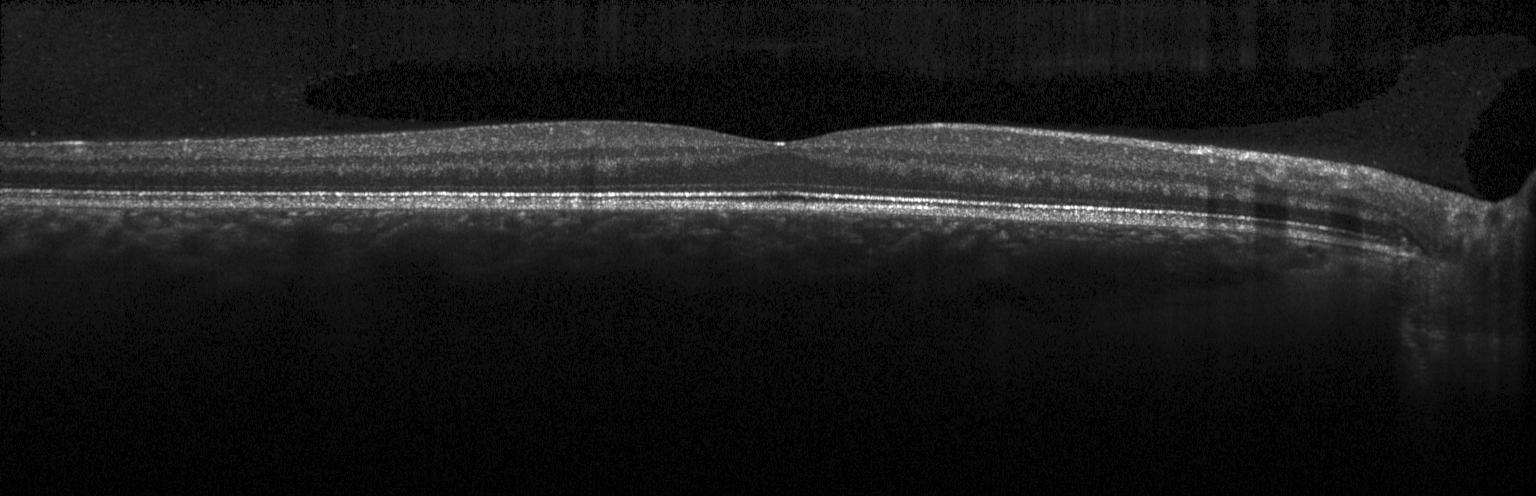

OCT finding: no evidence of choroidal neovascularization, diabetic macular edema, or drusen.